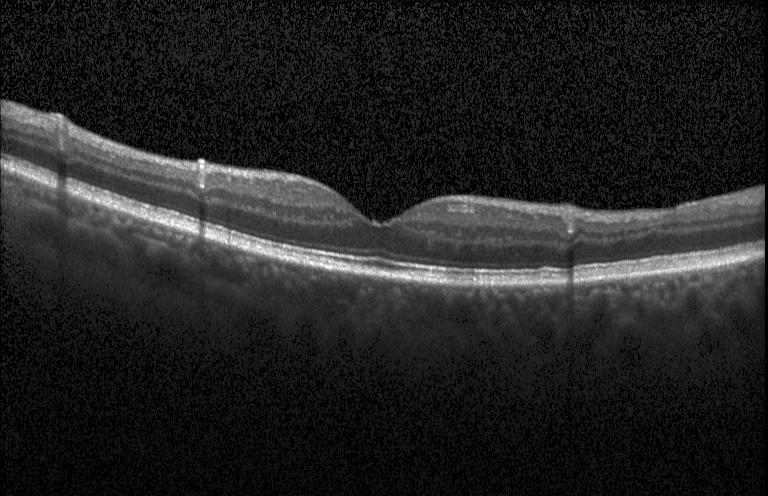
Retinal OCT cross-section · through the macula · acquired on a Heidelberg Spectralis
This B-scan demonstrates no choroidal neovascularization, no diabetic macular edema, and no drusen.